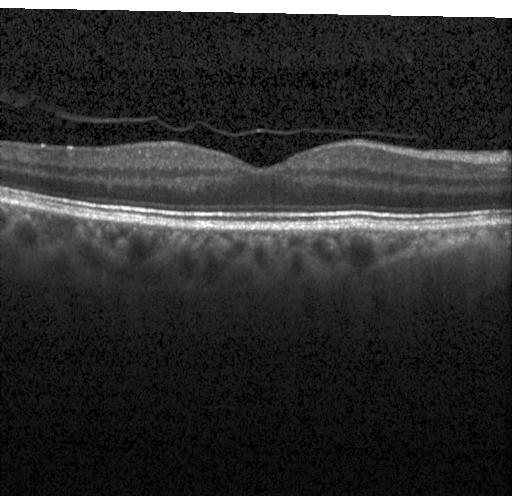

Fovea-centered · instrument: Heidelberg Spectralis · OCT line scan · spectral-domain OCT.
Dx: neither CNV, DME, nor drusen.